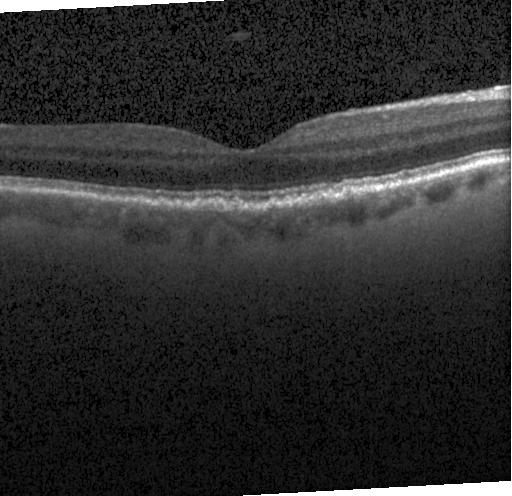 Optical coherence tomography B-scan · through the macula
OCT finding: drusen.